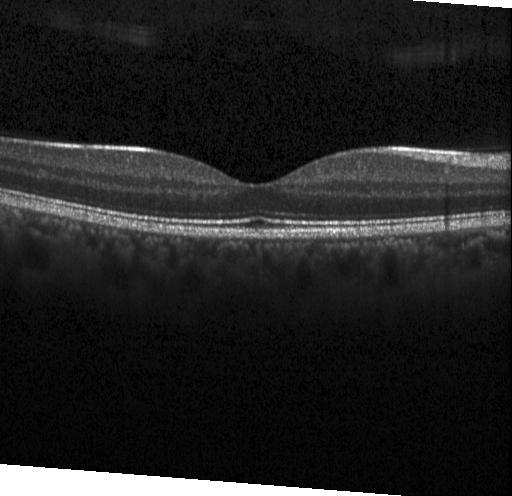

Dx: no choroidal neovascularization, no diabetic macular edema, and no drusen.